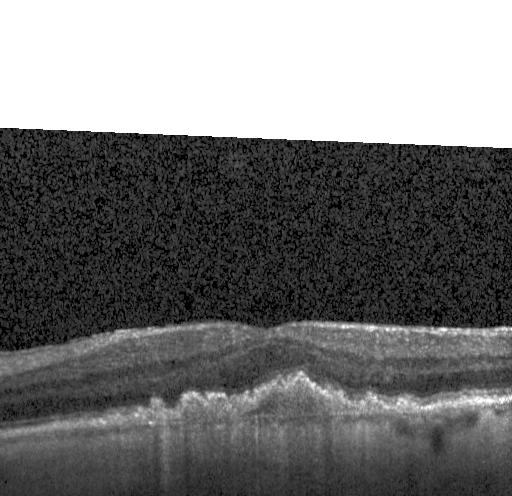

Optical coherence tomography scan. Diagnosis: choroidal neovascularization.